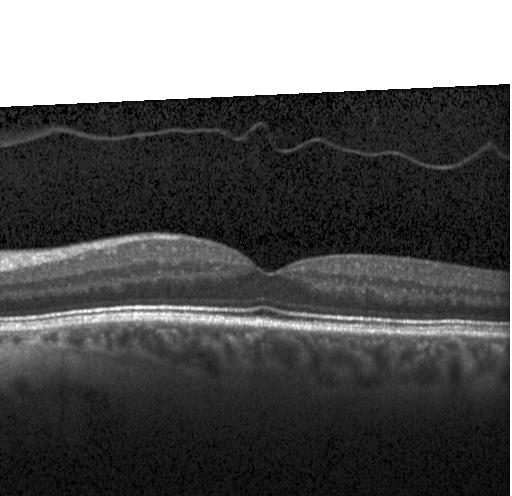 Retinal OCT B-scan — The scan shows no evidence of choroidal neovascularization, diabetic macular edema, or drusen.